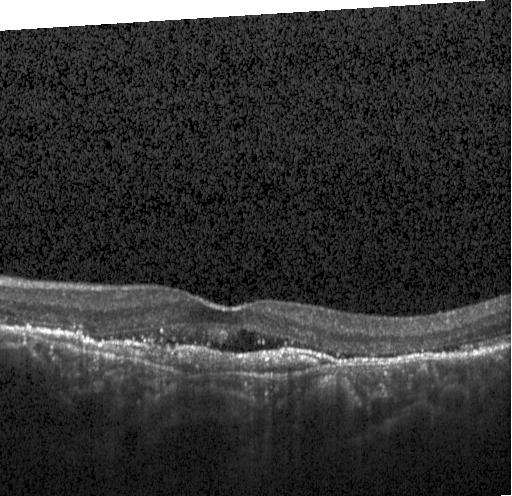
Heidelberg Spectralis; OCT B-scan; fovea-centered — Diagnosis: a choroidal neovascular membrane.